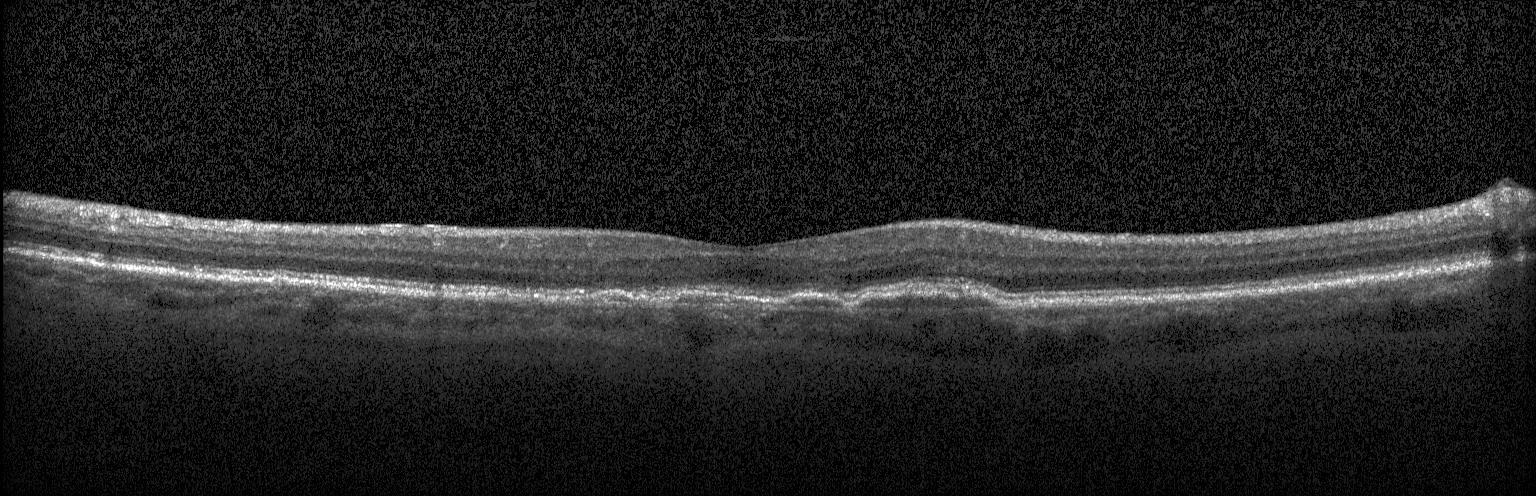 Heidelberg Spectralis; through the macula; OCT line scan — Impression: choroidal neovascularization.